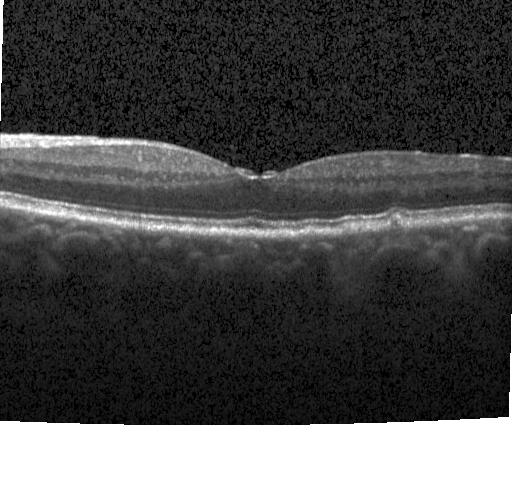 Optical coherence tomography scan. Diagnosis: multiple drusen.